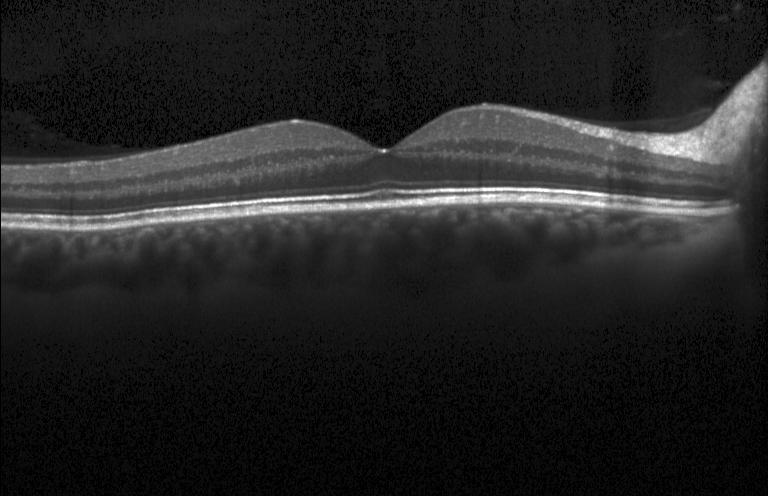

Spectral-domain OCT, acquired on a Heidelberg Spectralis, OCT line scan.
This B-scan demonstrates neither choroidal neovascularization, diabetic macular edema, nor drusen.